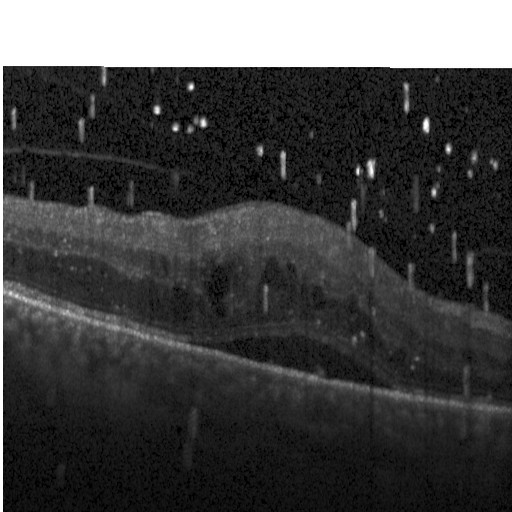

Retinal OCT cross-section · Heidelberg Spectralis
Assessment: DME.